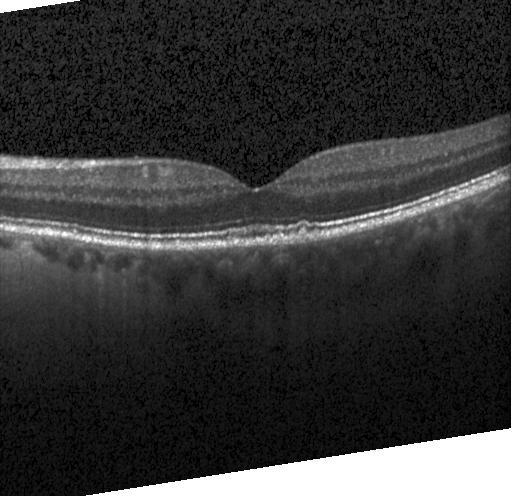 Optical coherence tomography B-scan
Diagnosis: multiple drusen.